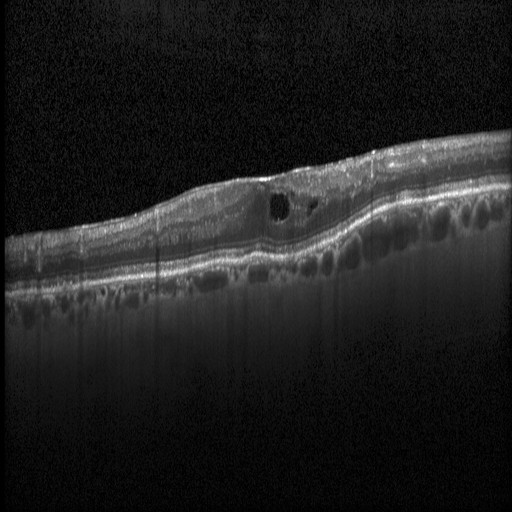 Retinal OCT cross-section, horizontal scan through the fovea — Finding: diabetic macular edema.